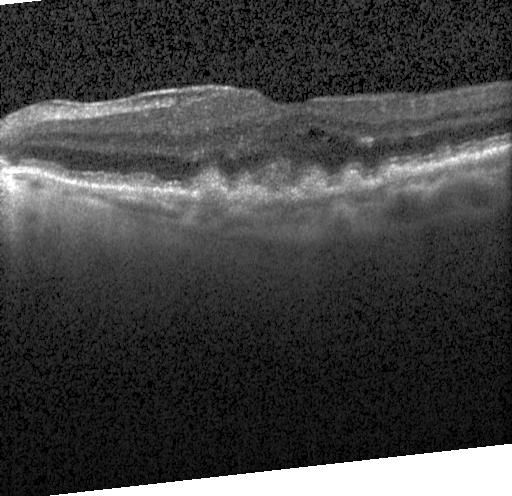 OCT line scan, SD-OCT — Macular OCT: choroidal neovascularization.